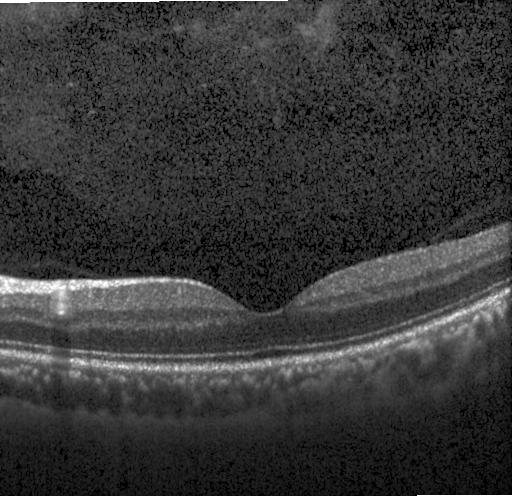 Instrument: Heidelberg Spectralis · retinal OCT cross-section — Diagnosis: neither choroidal neovascularization, diabetic macular edema, nor drusen.